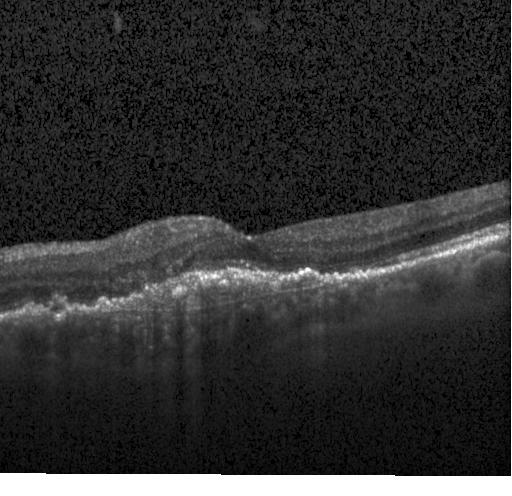 Centered on the fovea · spectral-domain OCT · retinal OCT B-scan. The scan shows choroidal neovascularization (CNV).